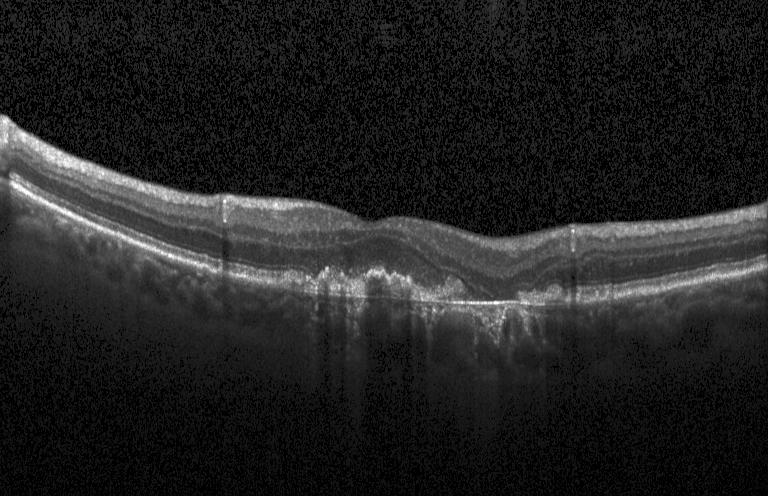
Diagnosis: CNV.